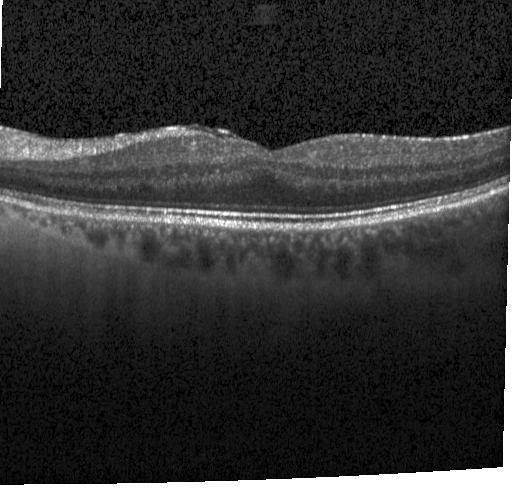 Retinal OCT cross-section · spectral-domain OCT · through the macula
Macular OCT: no evidence of CNV, DME, or drusen.